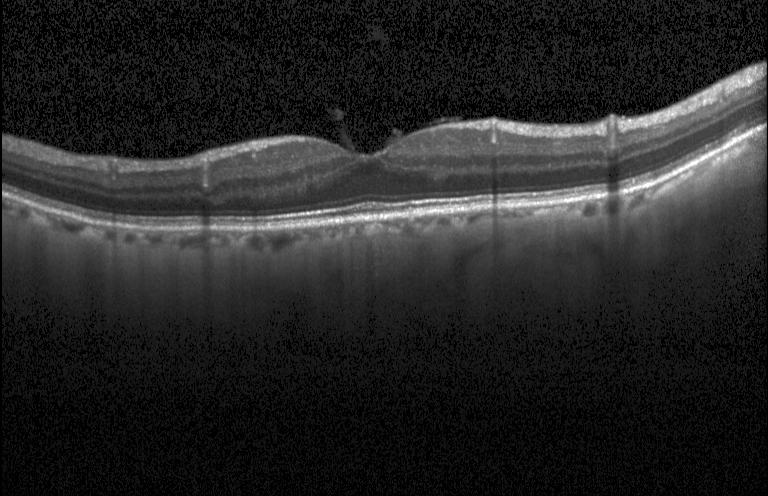

Retinal OCT B-scan
Impression: neither choroidal neovascularization, diabetic macular edema, nor drusen.